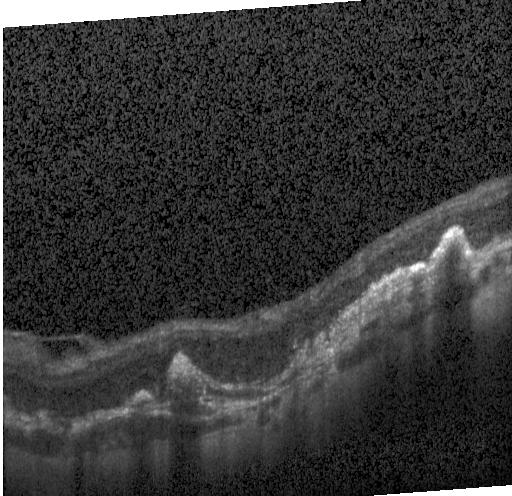

Optical coherence tomography B-scan, centered on the fovea, instrument: Heidelberg Spectralis
Diagnosis: CNV.